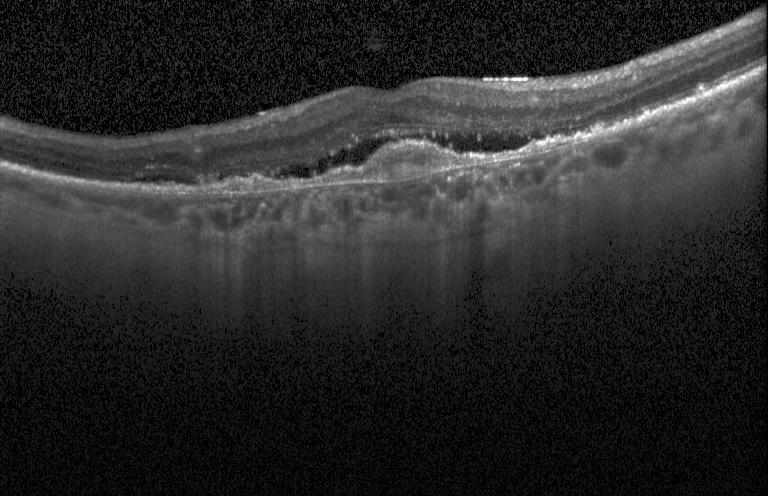
Impression: CNV.